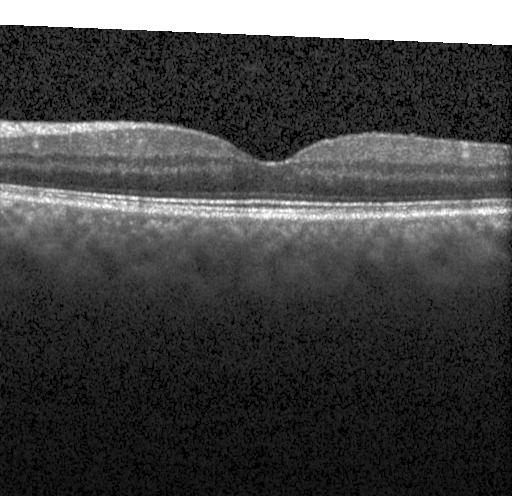
Retinal OCT cross-section. Spectral-domain OCT.
Dx: no choroidal neovascularization, diabetic macular edema, or drusen.